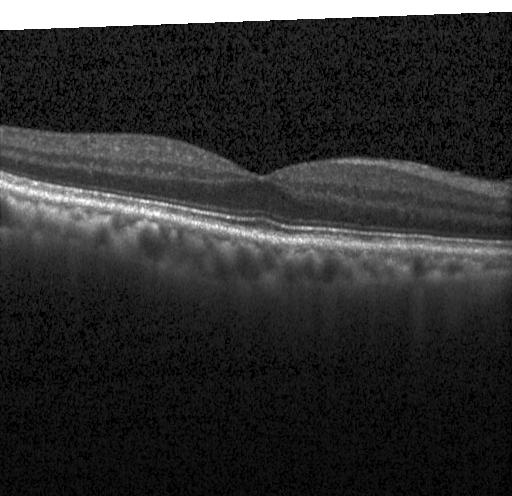
Spectral-domain OCT B-scan: no evidence of choroidal neovascularization, diabetic macular edema, or drusen.